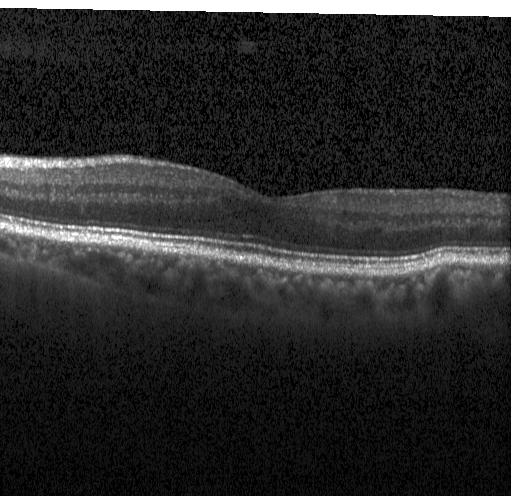

Finding: no choroidal neovascularization, diabetic macular edema, or drusen.